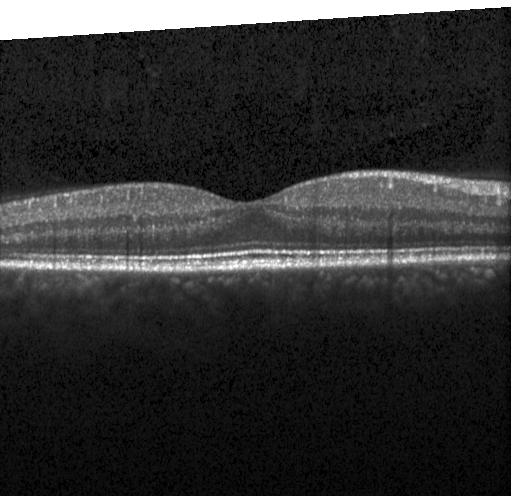
Heidelberg Spectralis. Spectral-domain optical coherence tomography. Fovea-centered. Optical coherence tomography B-scan.
Diagnosis: no choroidal neovascularization, no diabetic macular edema, and no drusen.